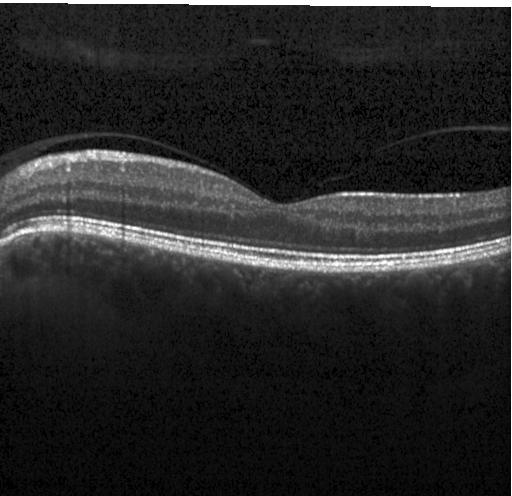 Retinal OCT cross-section. Heidelberg Spectralis OCT system. Spectral-domain optical coherence tomography. Fovea-centered.
Assessment: neither choroidal neovascularization, diabetic macular edema, nor drusen.